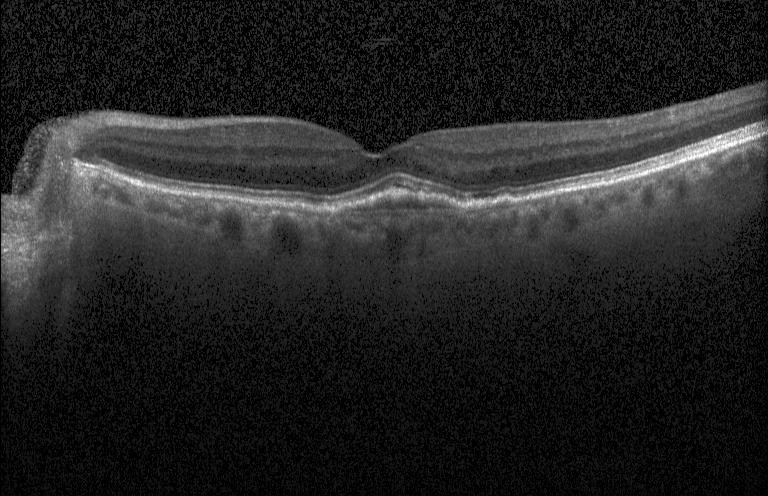

Spectral-domain OCT; optical coherence tomography scan. Finding: choroidal neovascularization (CNV).